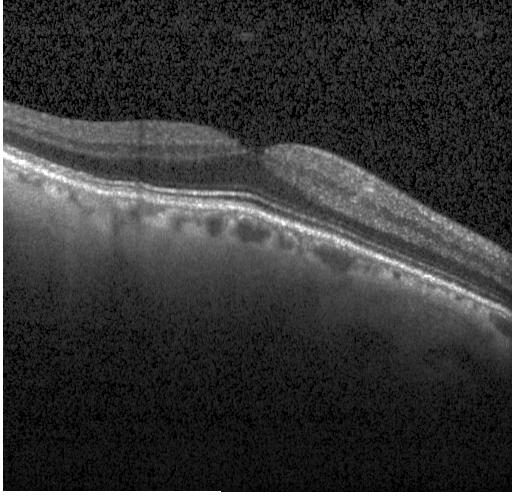

Retinal OCT B-scan; centered on the fovea
Assessment: no choroidal neovascularization, no diabetic macular edema, and no drusen.